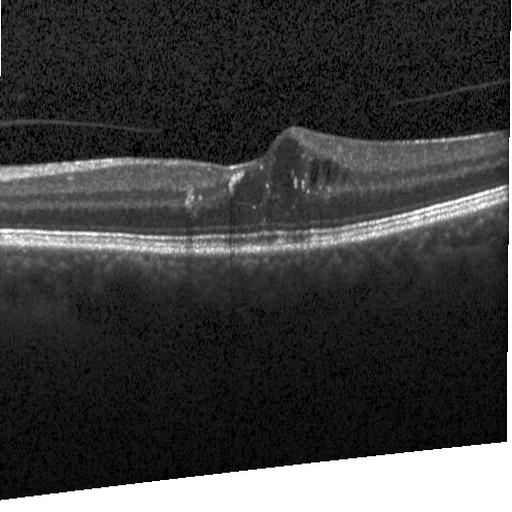

Spectral-domain optical coherence tomography. Macular scan. Retinal OCT cross-section.
Assessment: diabetic macular edema (DME).